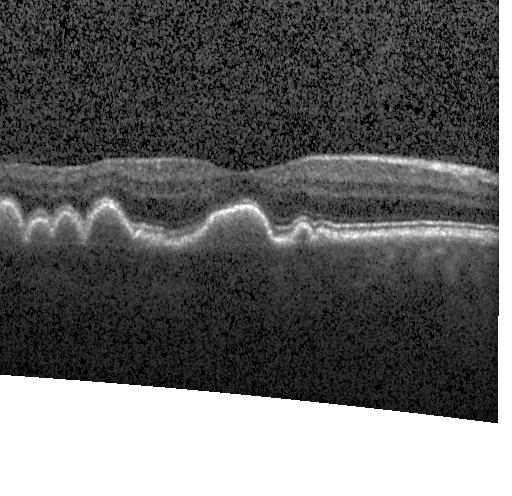 Dx: drusen.